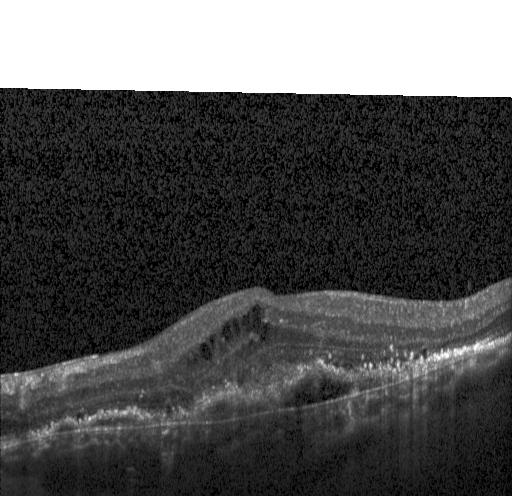 Heidelberg Spectralis, SD-OCT, OCT line scan, through the macula — Dx: choroidal neovascularization.